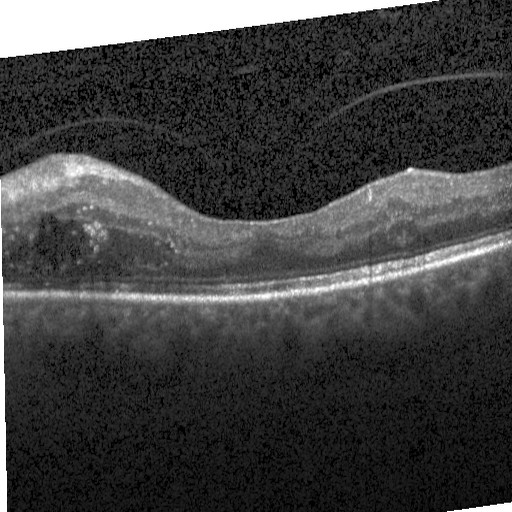
Macular scan. Retinal OCT B-scan — Macular OCT: diabetic macular edema (DME).